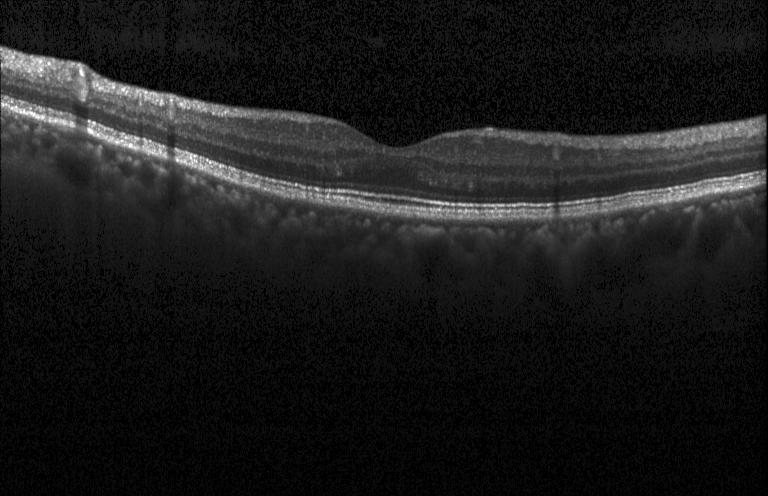 Acquired on a Heidelberg Spectralis · OCT line scan · macular scan · SD-OCT
Dx: no evidence of CNV, DME, or drusen.